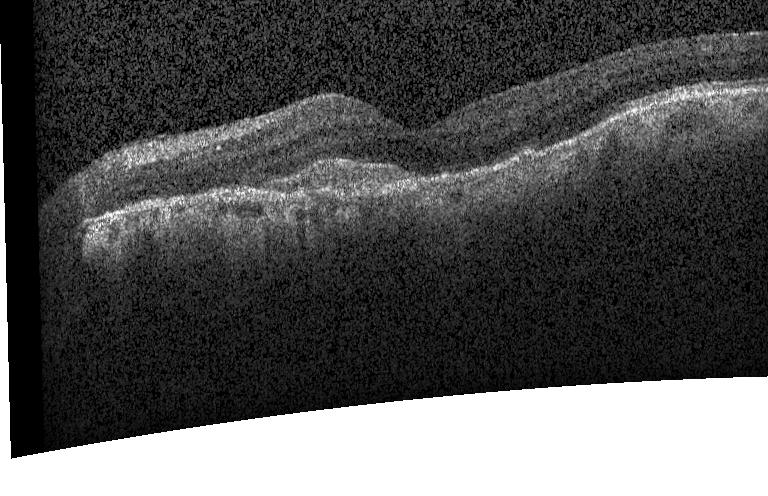

Spectral-domain OCT · Heidelberg Spectralis OCT system · OCT line scan · macular scan. The scan shows choroidal neovascularization.